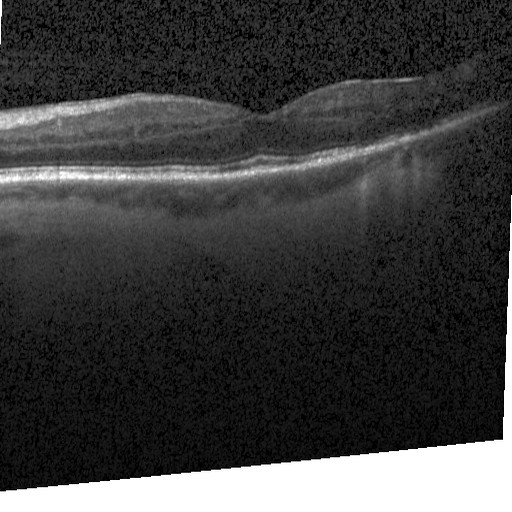

Acquired on a Heidelberg Spectralis; horizontal scan through the fovea; spectral-domain OCT; retinal OCT cross-section — Impression: diabetic macular edema (DME).